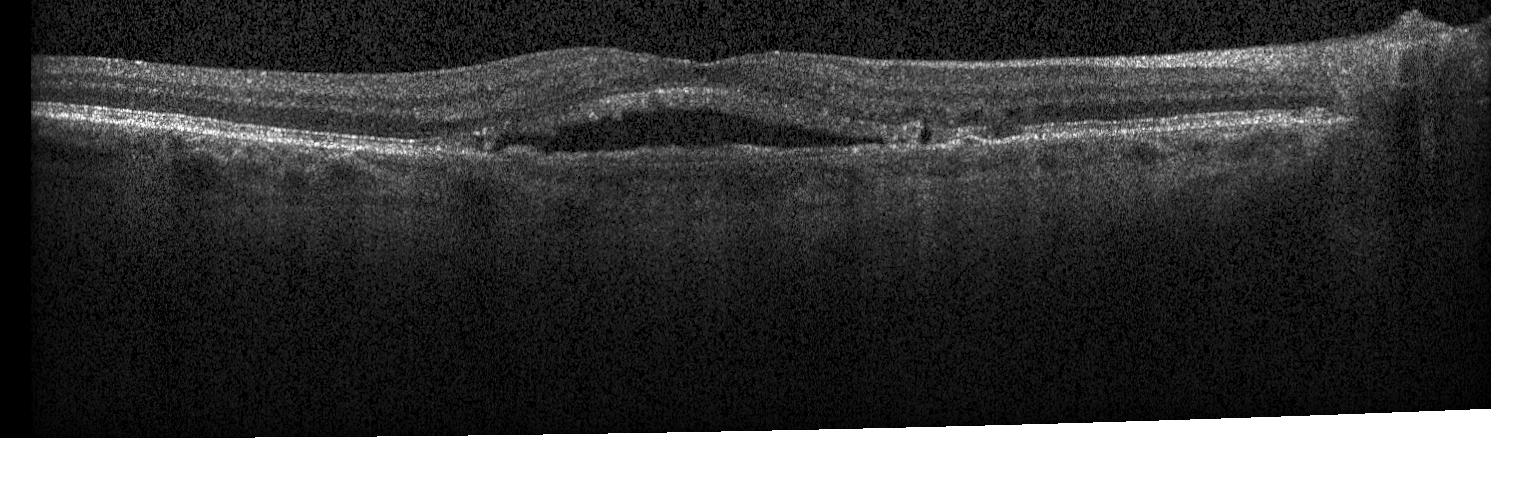 Retinal OCT B-scan, through the macula, spectral-domain OCT.
Assessment: a choroidal neovascular membrane.